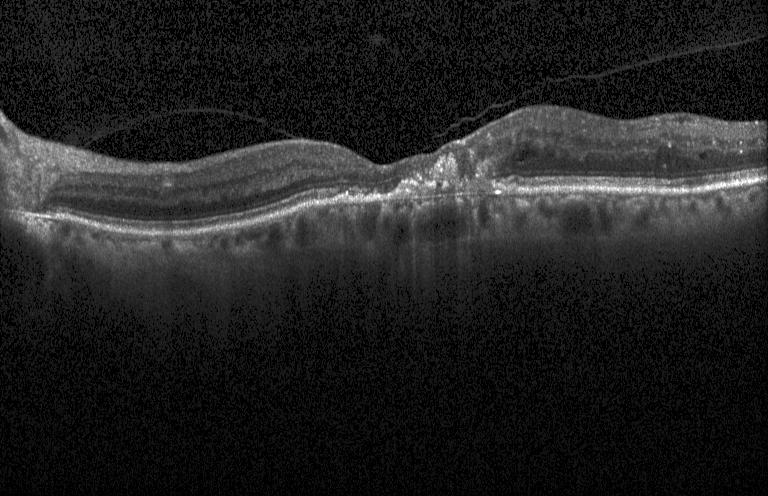 Heidelberg Spectralis OCT system; retinal OCT B-scan. Diagnosis: a choroidal neovascular membrane.